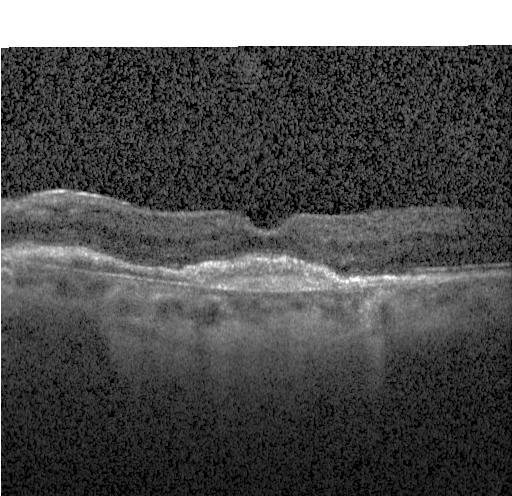 Spectral-domain optical coherence tomography · Heidelberg Spectralis · retinal OCT cross-section · macular scan
The scan shows a choroidal neovascular membrane.